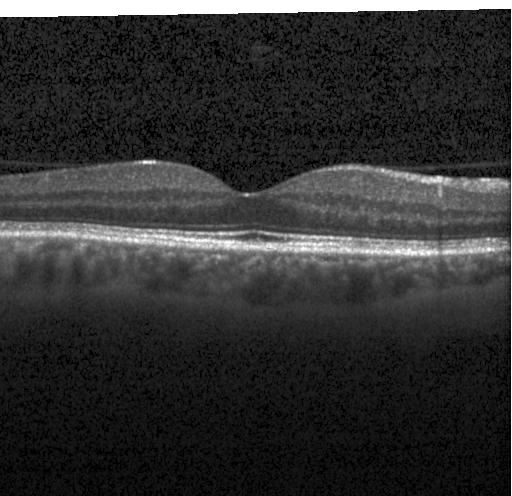 Spectral-domain OCT B-scan: no evidence of CNV, DME, or drusen.